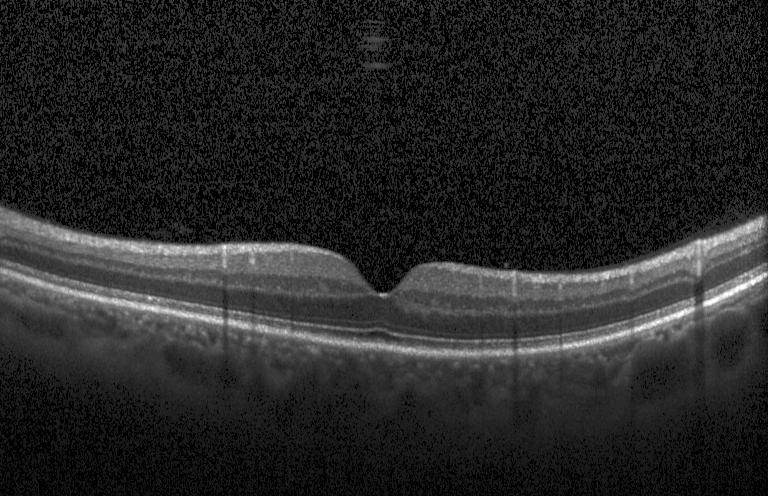
Retinal OCT B-scan, Heidelberg Spectralis, through the macula.
The scan shows no CNV, DME, or drusen.